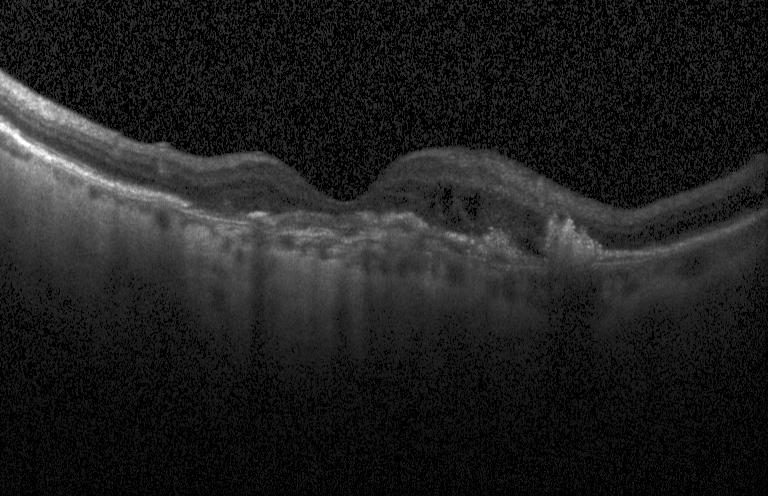

Optical coherence tomography B-scan — This B-scan demonstrates a choroidal neovascular membrane.